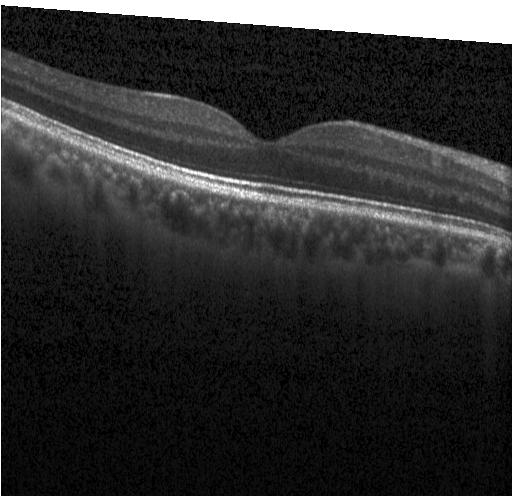

Diagnosis: no evidence of choroidal neovascularization, diabetic macular edema, or drusen.